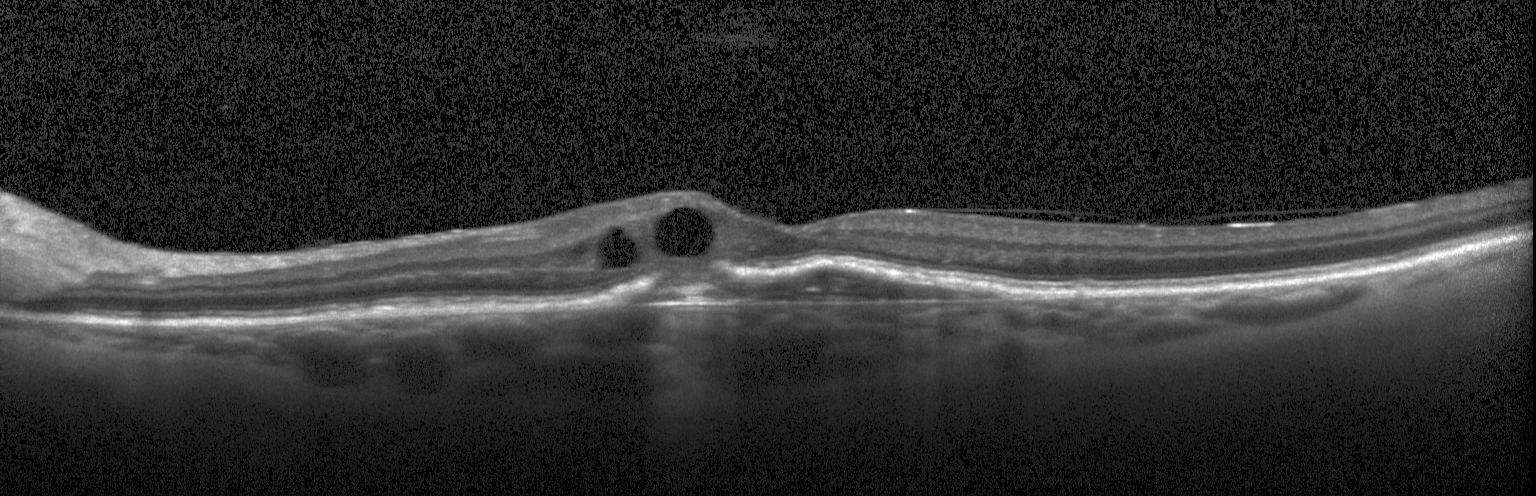

Retinal OCT cross-section; SD-OCT — Impression: a choroidal neovascular membrane.